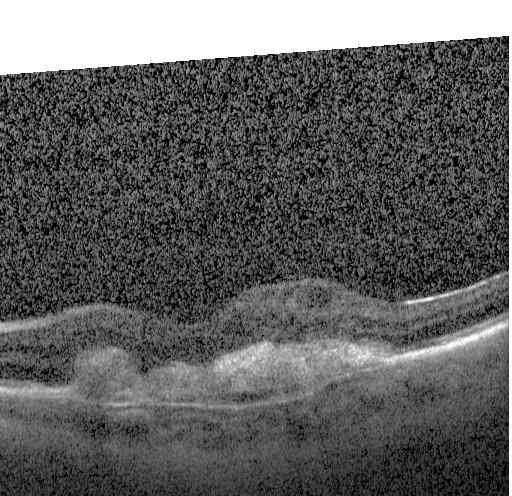
OCT B-scan showing a choroidal neovascular membrane.